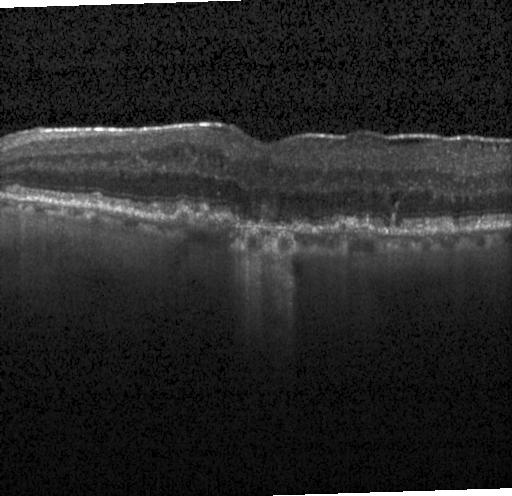

Retinal OCT B-scan. Macular scan. Spectral-domain OCT. Acquired on a Heidelberg Spectralis.
Diagnosis: a choroidal neovascular membrane.